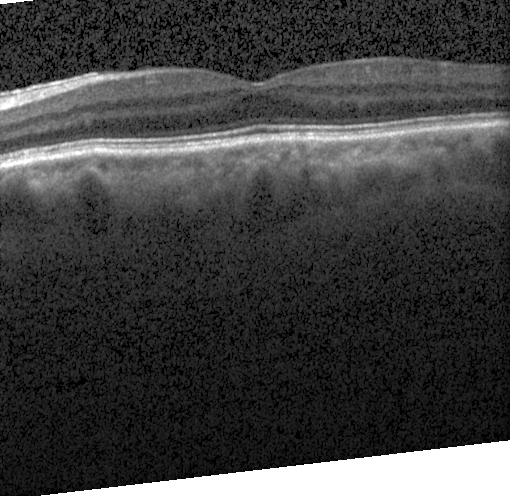
Heidelberg Spectralis OCT system · optical coherence tomography scan · macular scan · spectral-domain OCT.
Impression: no evidence of CNV, DME, or drusen.